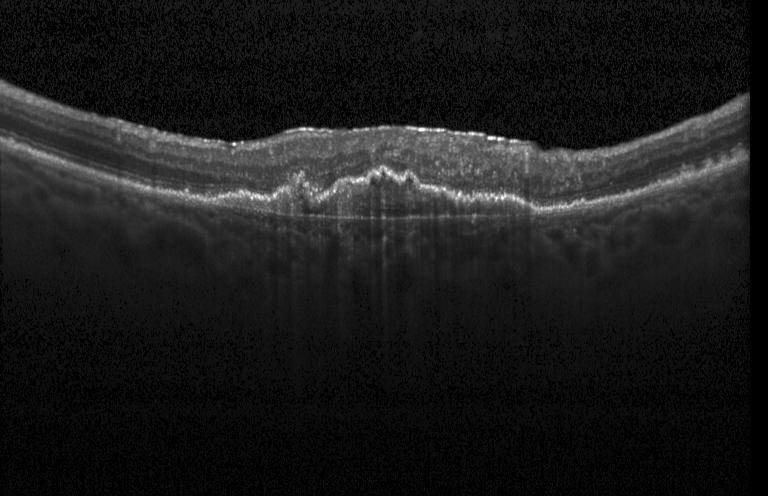 Impression: a choroidal neovascular membrane.